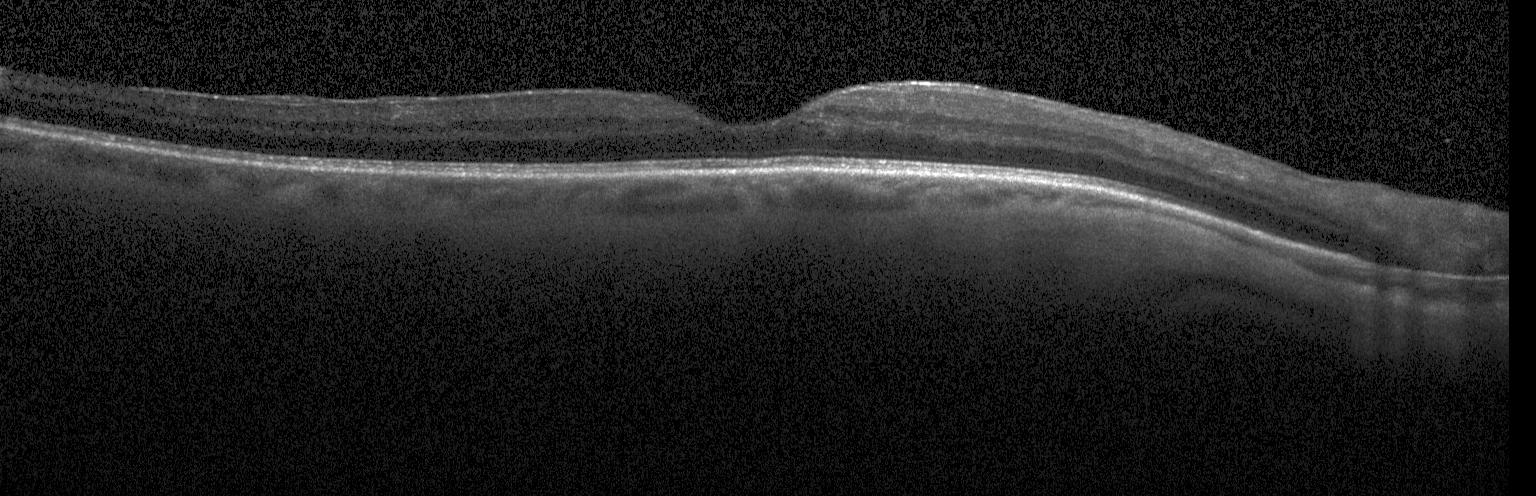
Heidelberg Spectralis OCT system; optical coherence tomography scan; SD-OCT; centered on the fovea
No choroidal neovascularization, diabetic macular edema, or drusen.